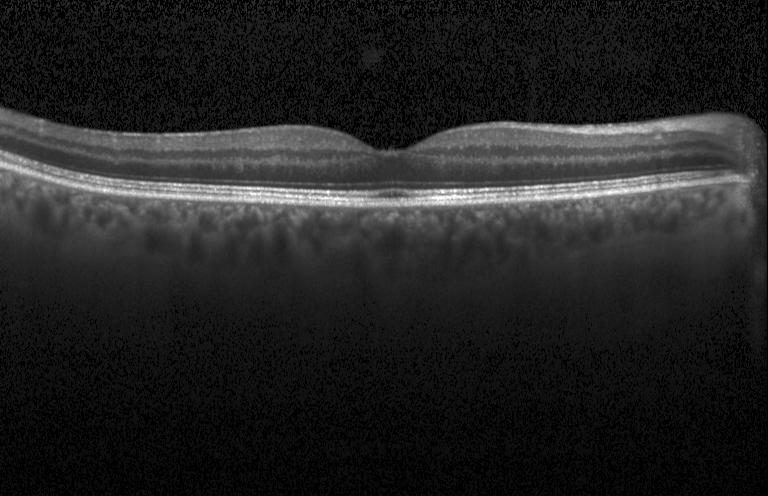
Macular OCT: no choroidal neovascularization, no diabetic macular edema, and no drusen.